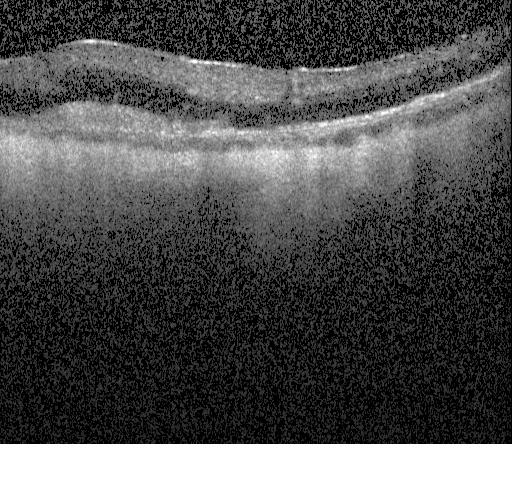
OCT line scan. Heidelberg Spectralis. SD-OCT. Macular scan.
Macular OCT: choroidal neovascularization.